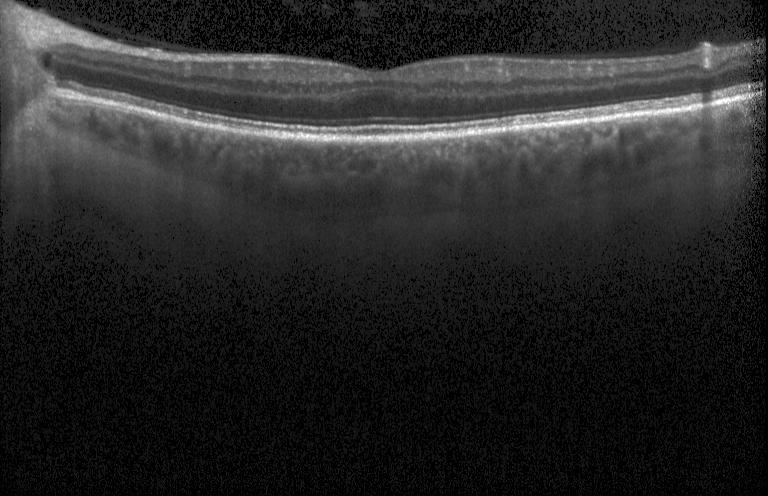 Finding: no evidence of choroidal neovascularization, diabetic macular edema, or drusen.